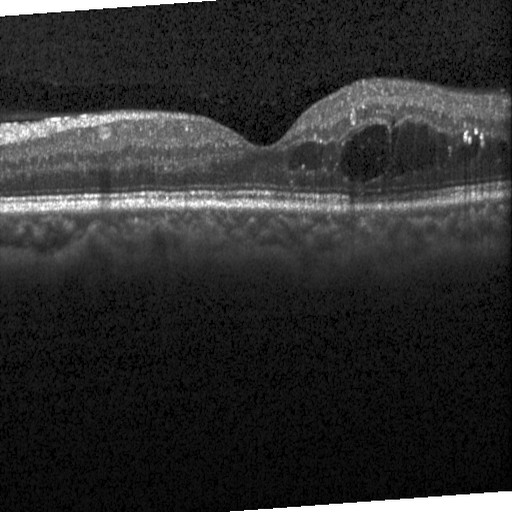

Diagnosis: DME.